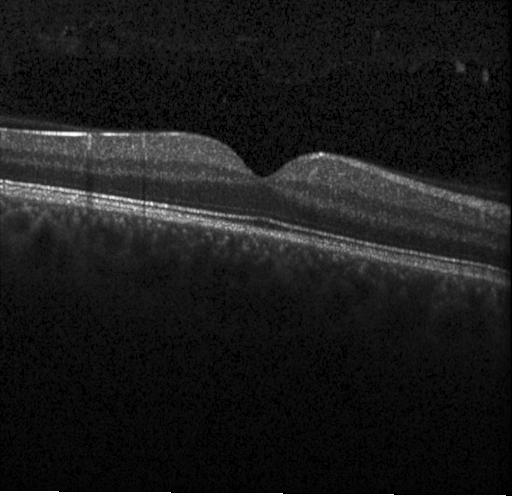 Spectral-domain OCT B-scan: no choroidal neovascularization, diabetic macular edema, or drusen.